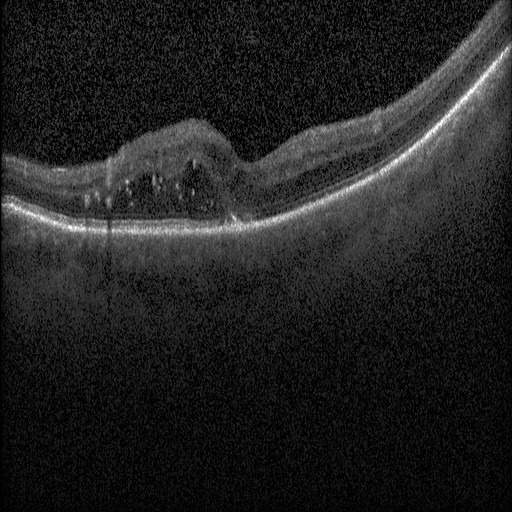
Spectral-domain optical coherence tomography, acquired on a Heidelberg Spectralis, OCT B-scan — Dx: diabetic macular edema (DME).